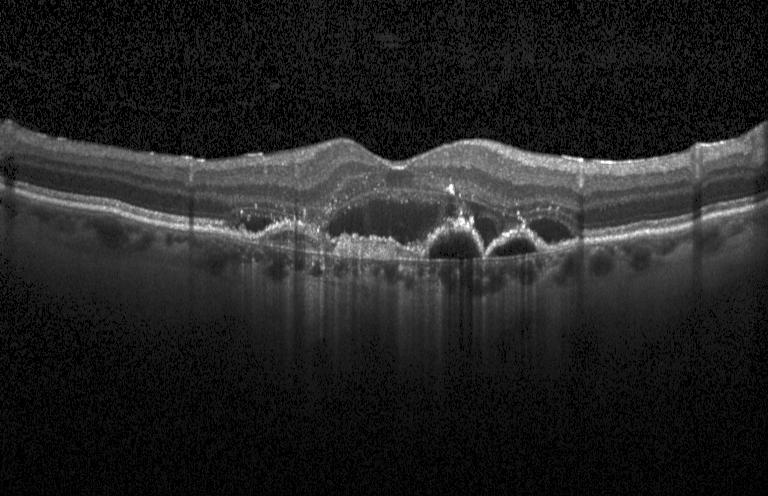

Macular scan, OCT line scan, acquired on a Heidelberg Spectralis — A choroidal neovascular membrane.